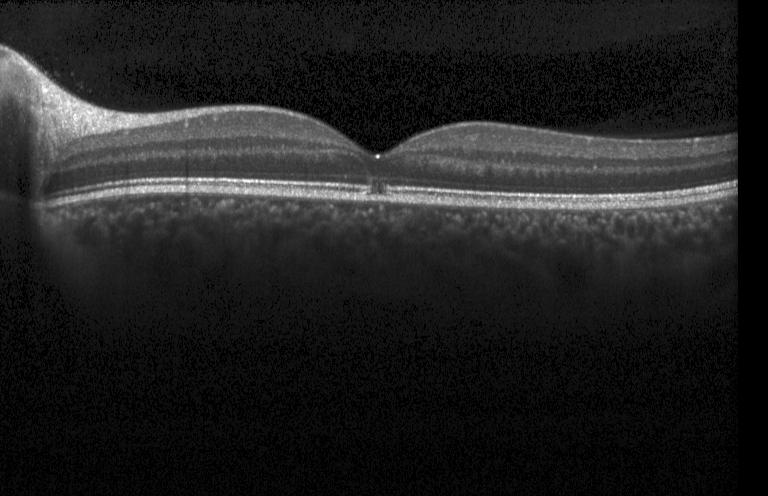 Finding: no CNV, DME, or drusen.